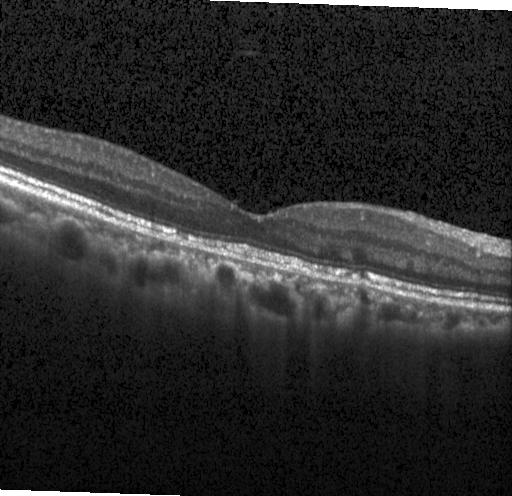

Horizontal scan through the fovea · retinal OCT B-scan · Heidelberg Spectralis OCT system · SD-OCT
Diagnosis: no choroidal neovascularization, diabetic macular edema, or drusen.